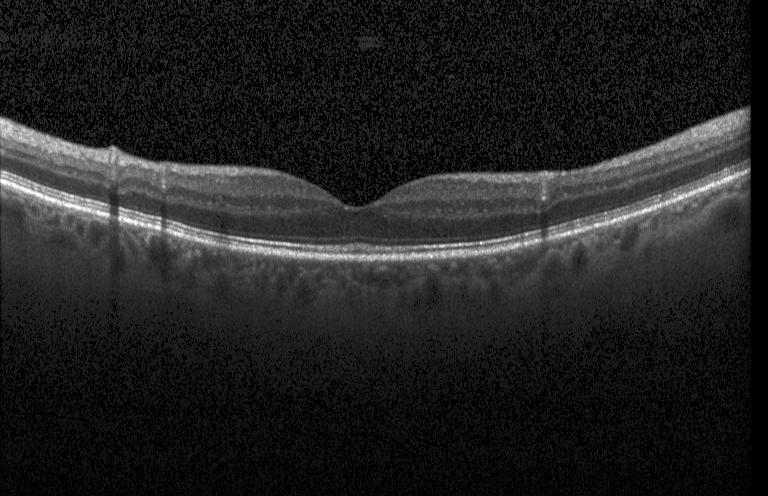

Finding: no choroidal neovascularization, no diabetic macular edema, and no drusen.